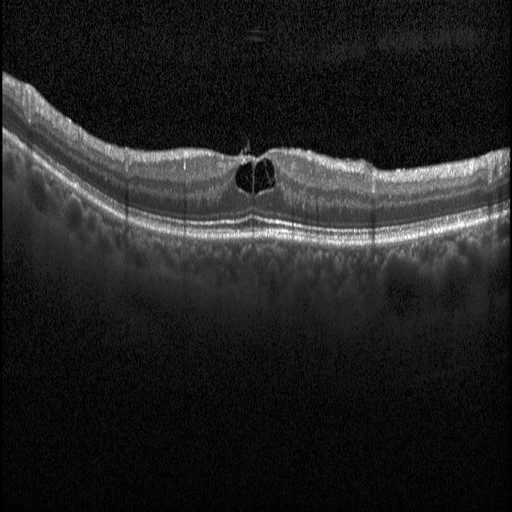
Diagnosis: diabetic macular edema (DME).